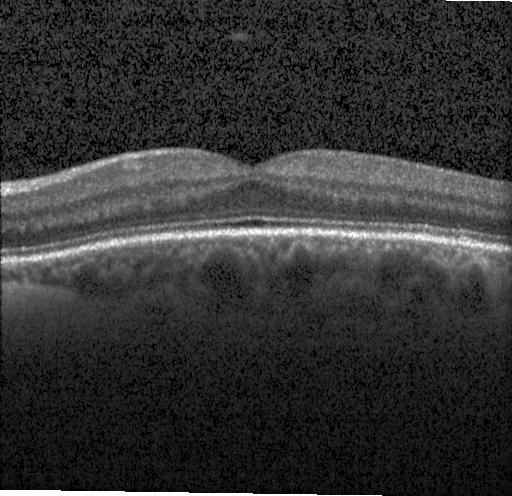 Macular scan · OCT B-scan · spectral-domain optical coherence tomography · Heidelberg Spectralis.
Macular OCT: neither CNV, DME, nor drusen.